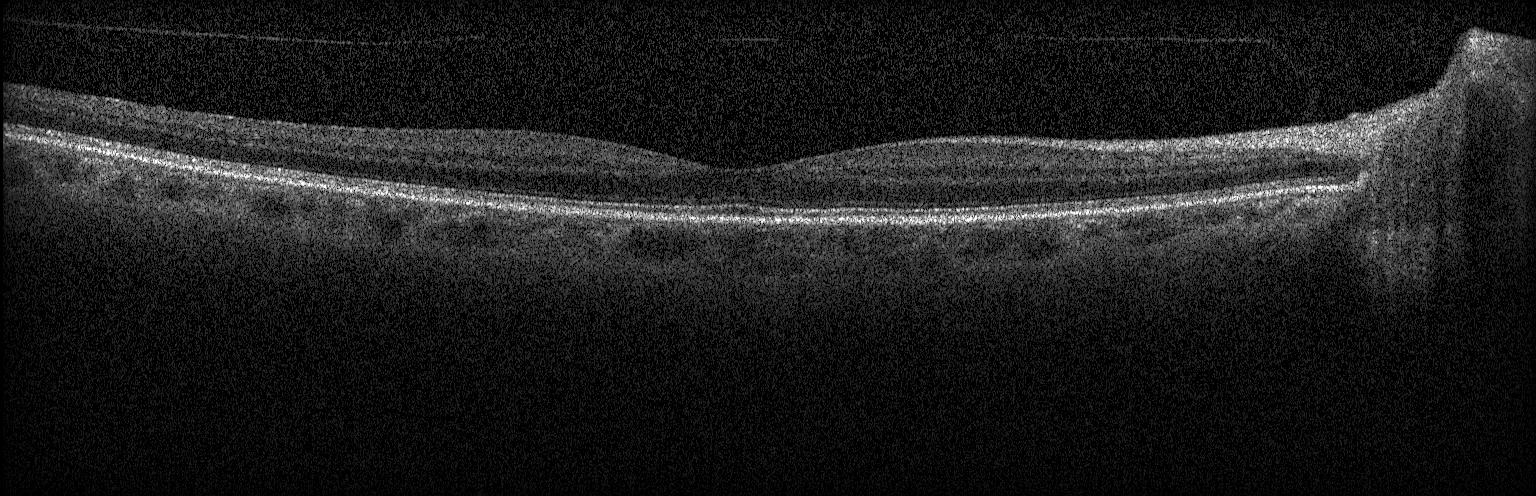 Heidelberg Spectralis, spectral-domain optical coherence tomography, optical coherence tomography scan, fovea-centered — Diagnosis: no CNV, no DME, and no drusen.